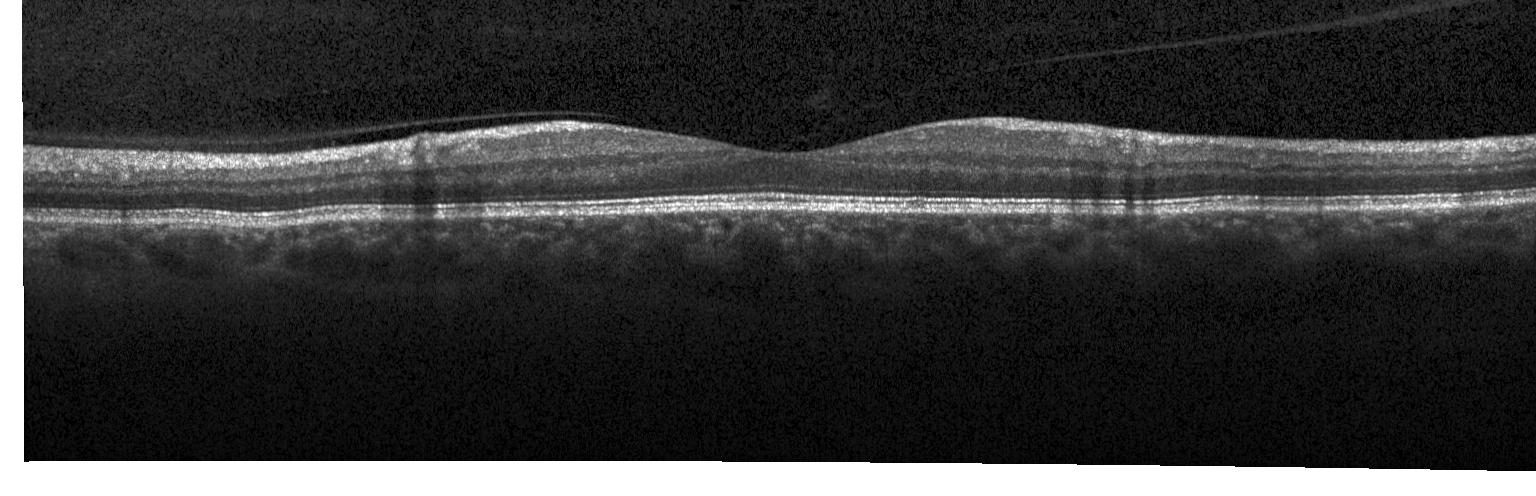
Impression: no CNV, DME, or drusen.